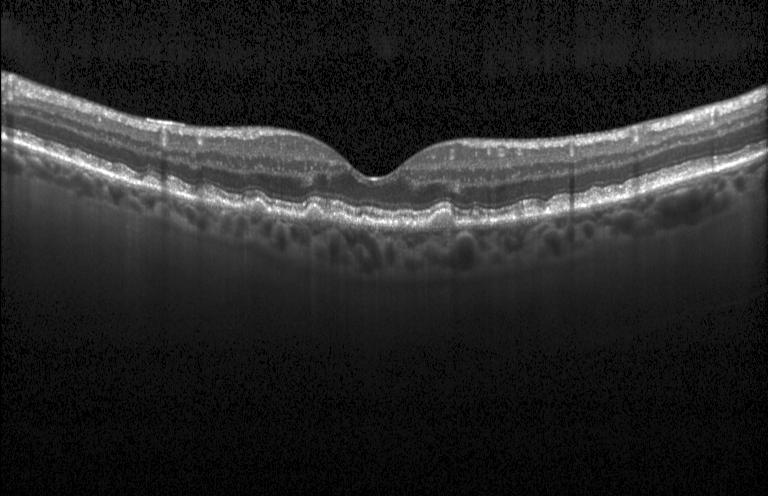
OCT finding: drusen.